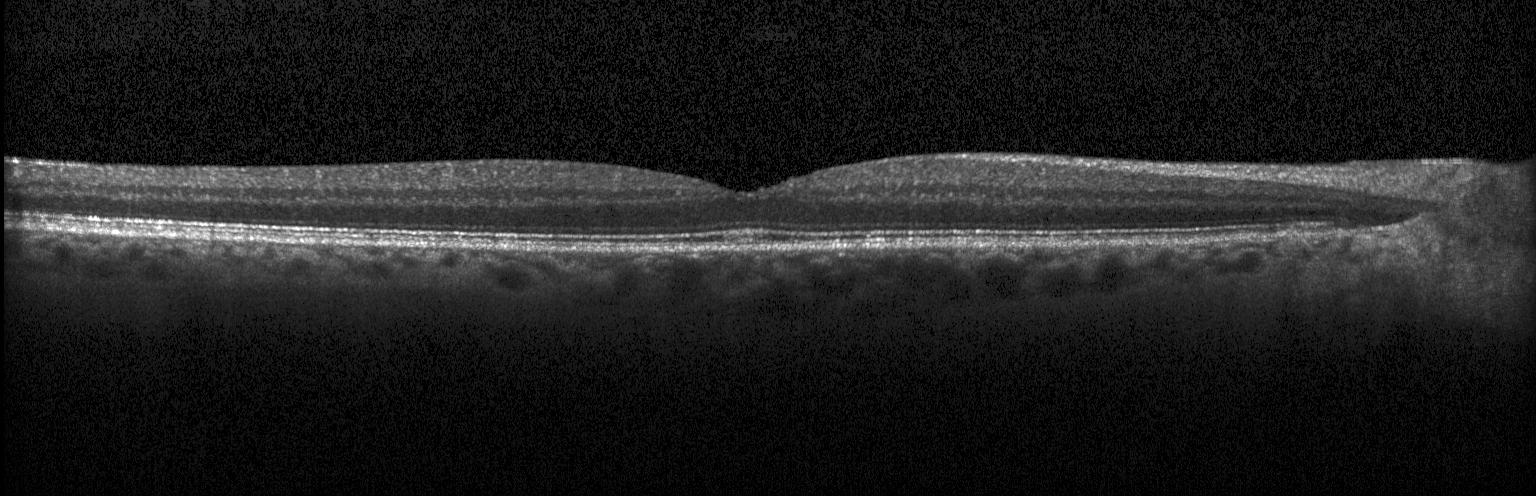
OCT B-scan — Macular OCT: neither choroidal neovascularization, diabetic macular edema, nor drusen.